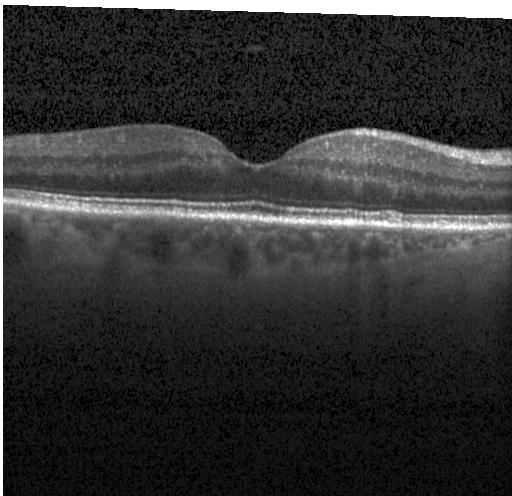

OCT finding: no choroidal neovascularization, no diabetic macular edema, and no drusen.